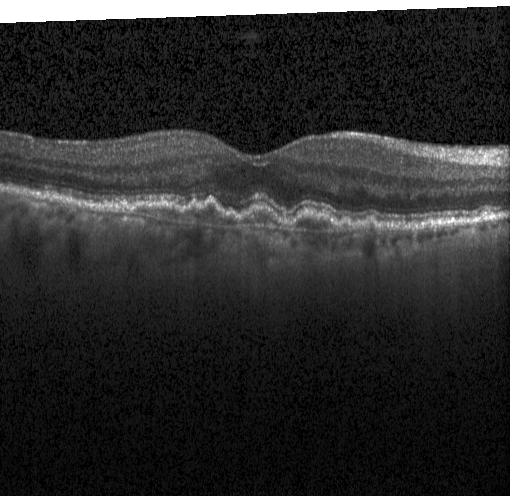
Horizontal scan through the fovea. Acquired on a Heidelberg Spectralis. Retinal OCT cross-section — This B-scan demonstrates a choroidal neovascular membrane.